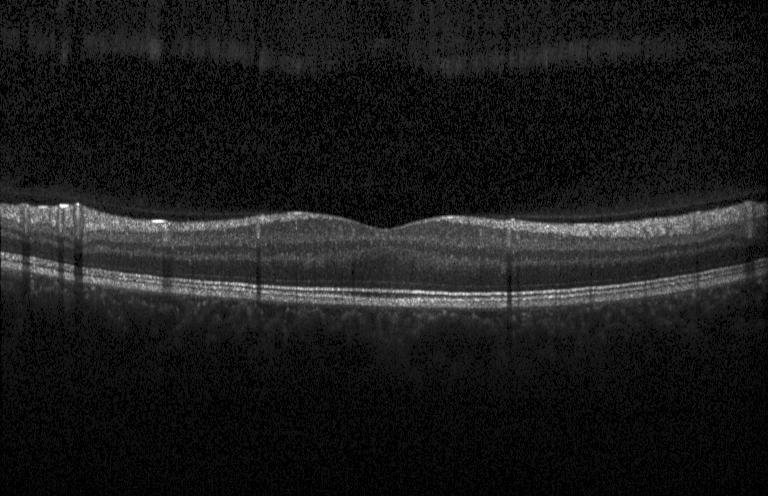
Impression: neither choroidal neovascularization, diabetic macular edema, nor drusen.